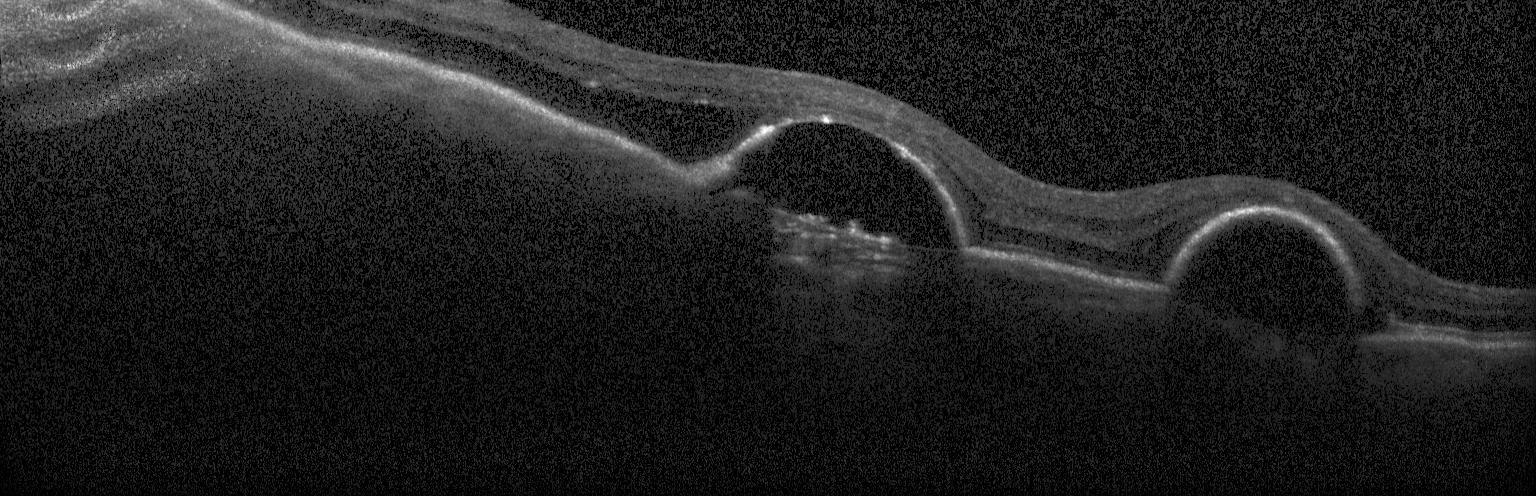
Finding: a choroidal neovascular membrane.